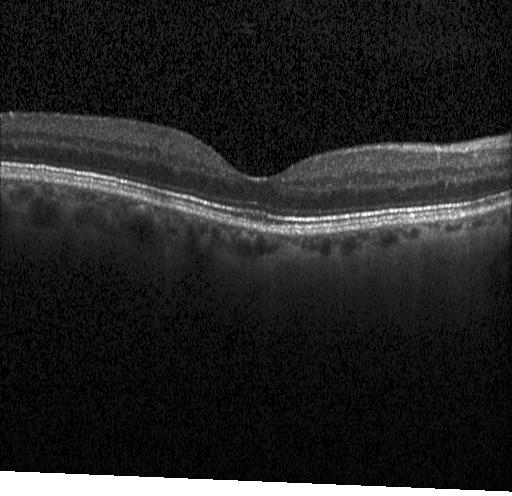 SD-OCT; optical coherence tomography B-scan; Heidelberg Spectralis OCT system; centered on the fovea. Impression: neither choroidal neovascularization, diabetic macular edema, nor drusen.